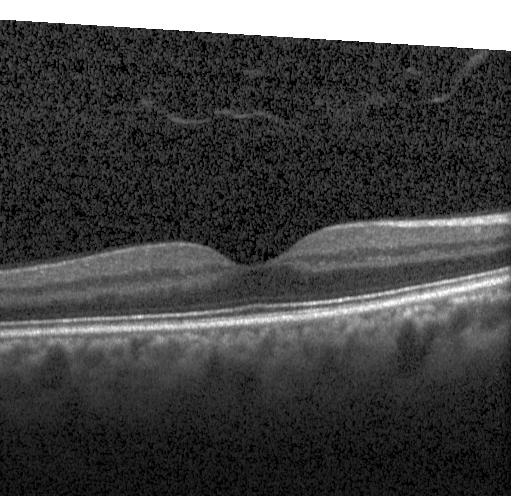

Finding: neither choroidal neovascularization, diabetic macular edema, nor drusen.